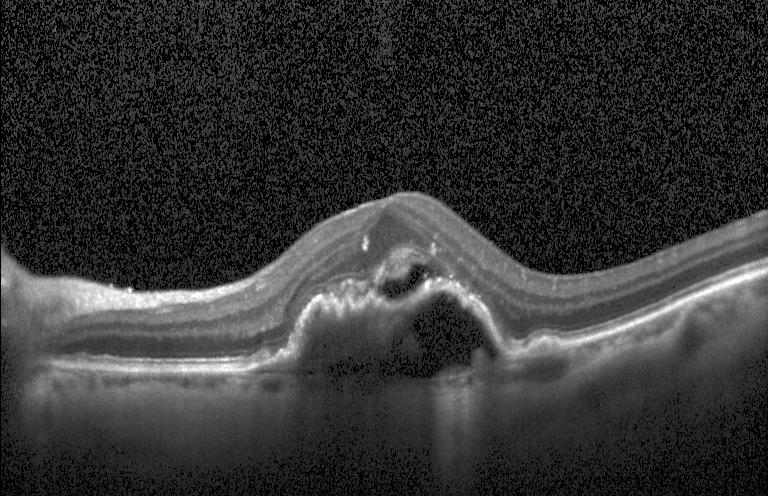 Retinal OCT B-scan
This B-scan demonstrates a choroidal neovascular membrane.